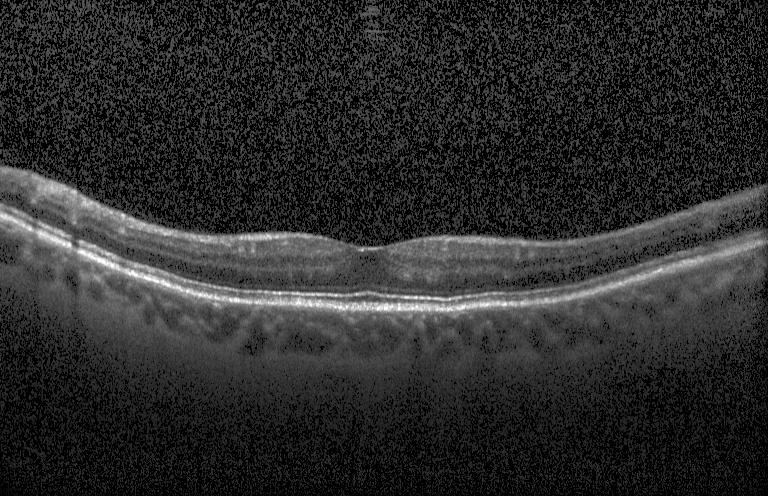
Spectral-domain OCT. Fovea-centered. Retinal OCT B-scan. Acquired on a Heidelberg Spectralis.
Macular OCT: no choroidal neovascularization, no diabetic macular edema, and no drusen.